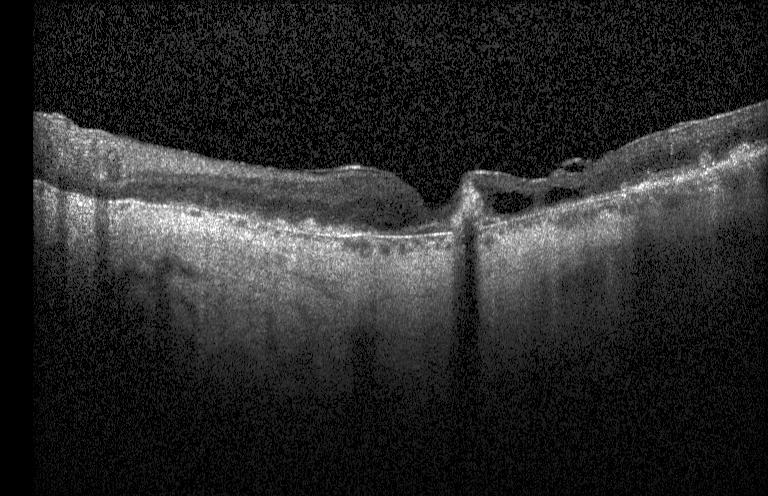 Macular OCT: a choroidal neovascular membrane.